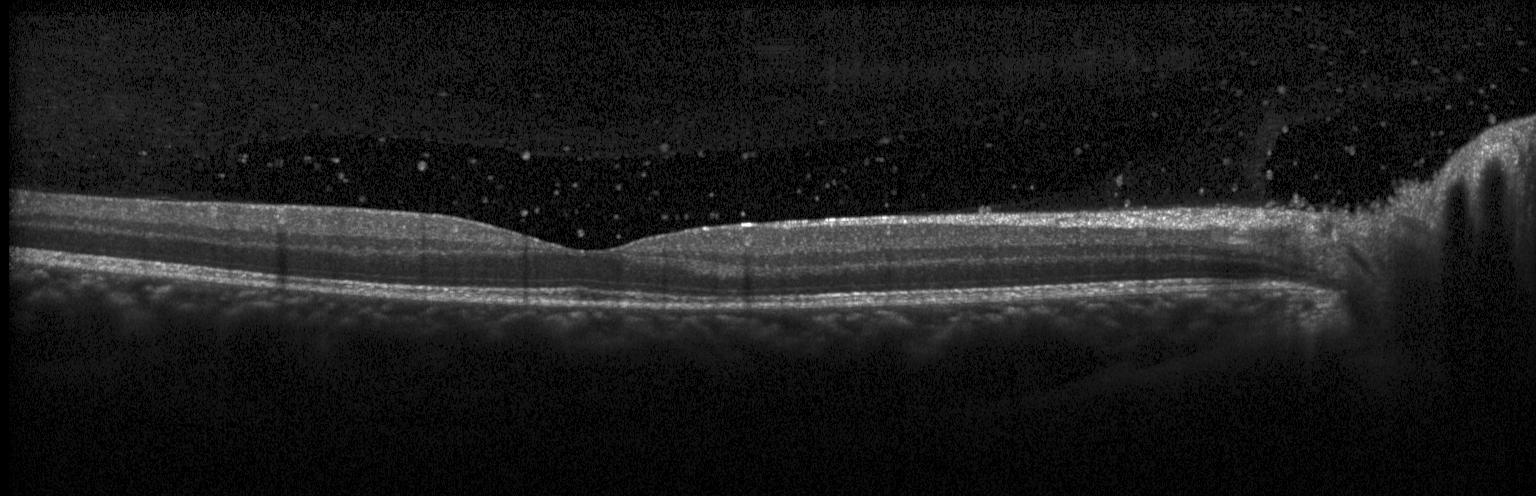 Assessment: no choroidal neovascularization, diabetic macular edema, or drusen.